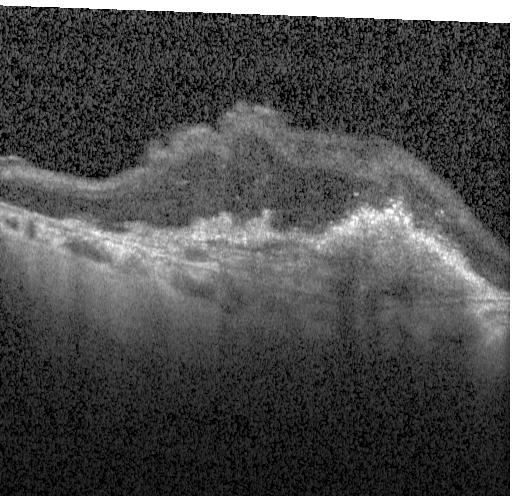

Finding: a choroidal neovascular membrane.